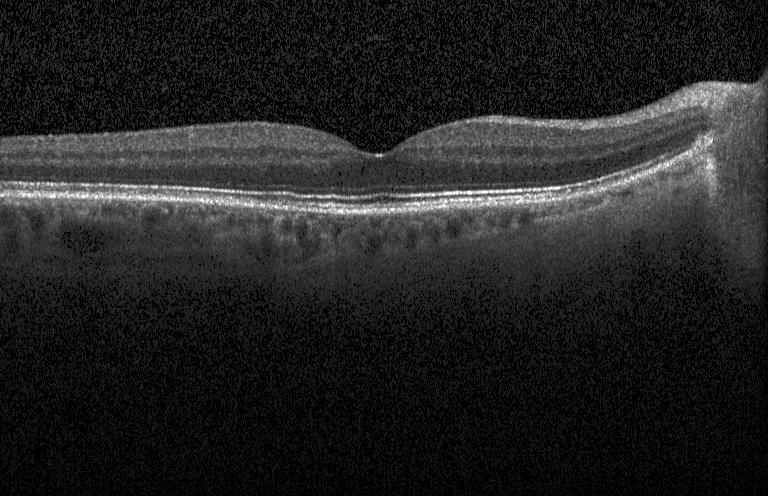
Macular OCT demonstrating no CNV, no DME, and no drusen.